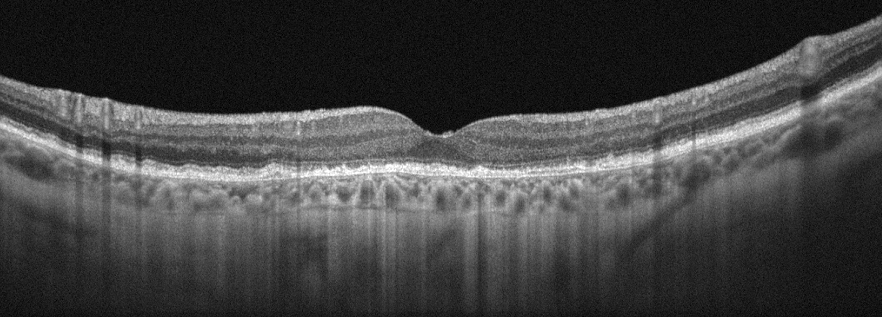
Optical coherence tomography B-scan · OD. The scan shows AMD.